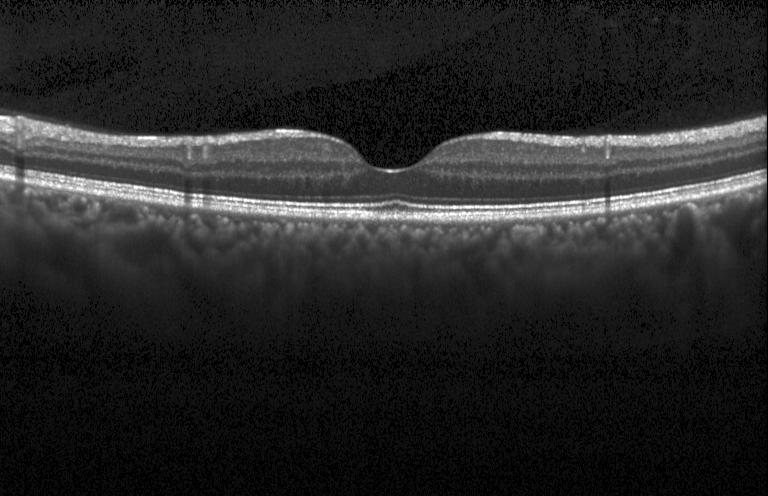 Centered on the fovea. OCT B-scan
Finding: no choroidal neovascularization, no diabetic macular edema, and no drusen.